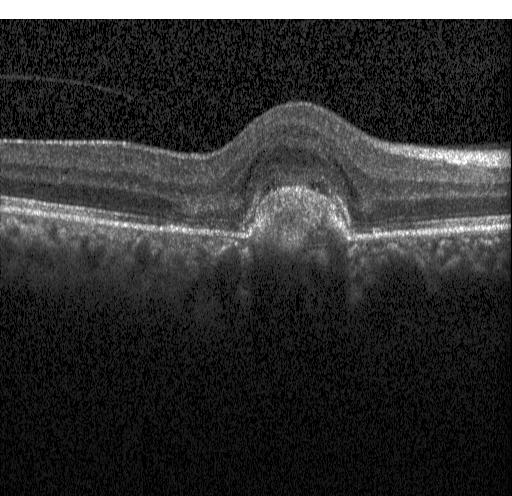 This B-scan demonstrates a choroidal neovascular membrane.